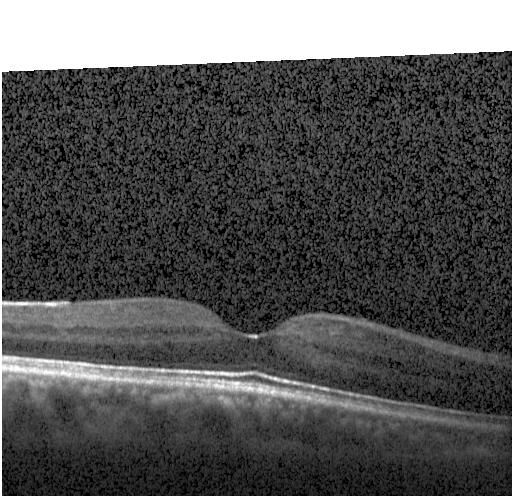

Spectral-domain OCT, retinal OCT cross-section — Impression: neither choroidal neovascularization, diabetic macular edema, nor drusen.